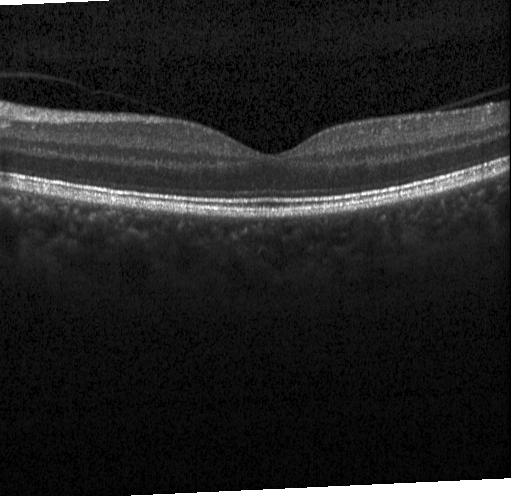 OCT line scan.
Diagnosis: no evidence of choroidal neovascularization, diabetic macular edema, or drusen.